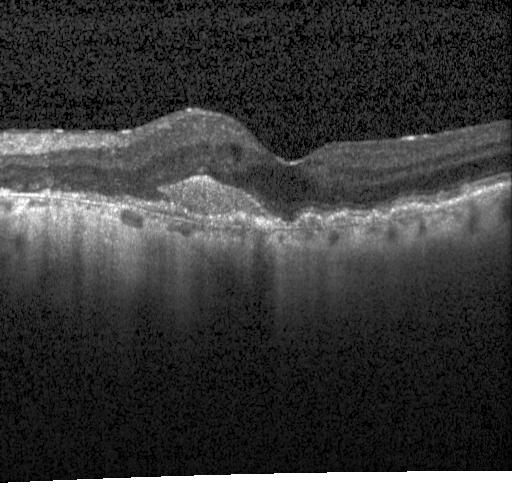
Spectral-domain OCT · optical coherence tomography B-scan · fovea-centered
The scan shows a choroidal neovascular membrane.